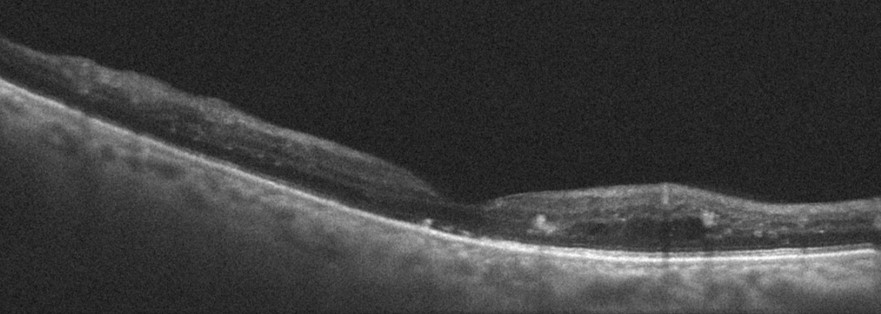

DME.